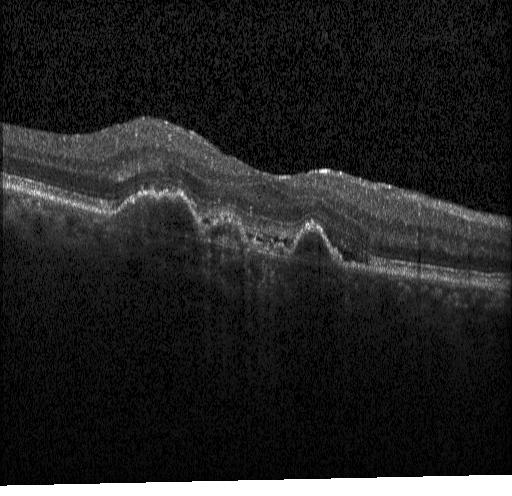
Optical coherence tomography scan
Finding: choroidal neovascularization (CNV).